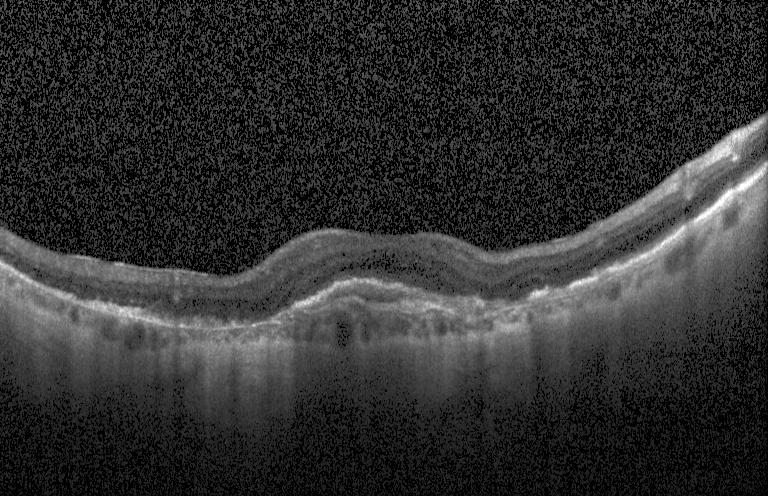
The scan shows choroidal neovascularization (CNV).